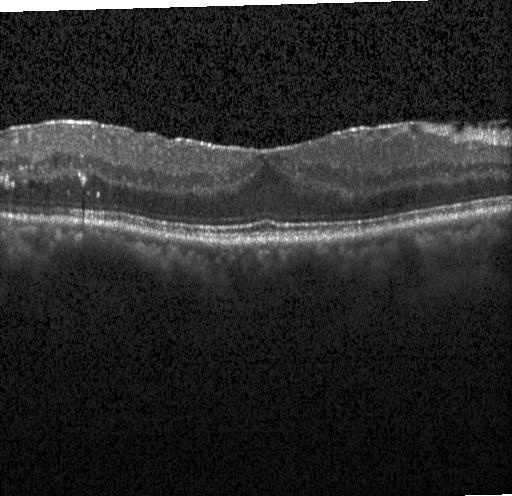

OCT line scan. Fovea-centered. Heidelberg Spectralis OCT system. Spectral-domain OCT. This B-scan demonstrates diabetic macular edema (DME).